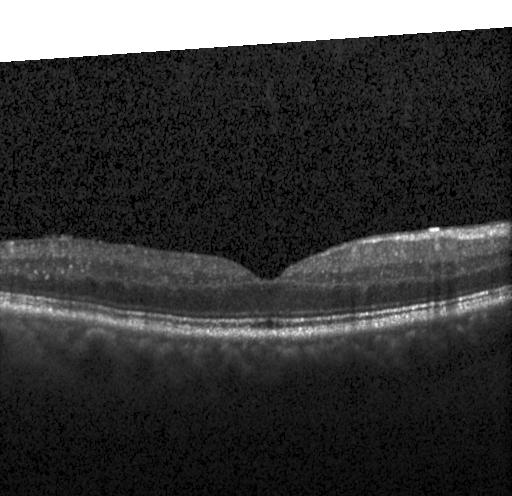

Neither choroidal neovascularization, diabetic macular edema, nor drusen.